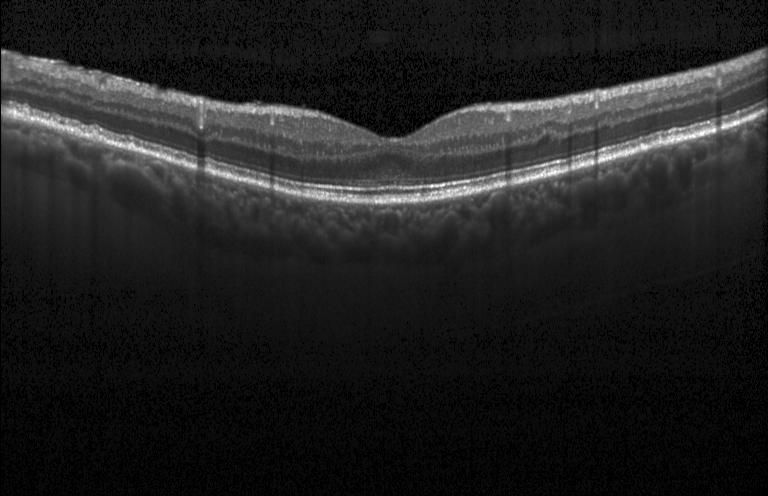 Macular OCT demonstrating no CNV, no DME, and no drusen.